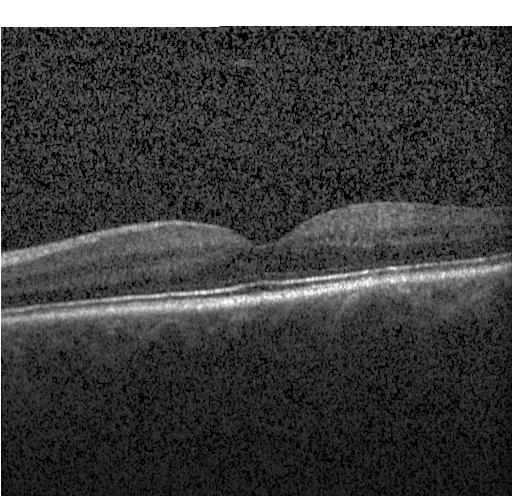
Optical coherence tomography B-scan, centered on the fovea. Diagnosis: neither choroidal neovascularization, diabetic macular edema, nor drusen.